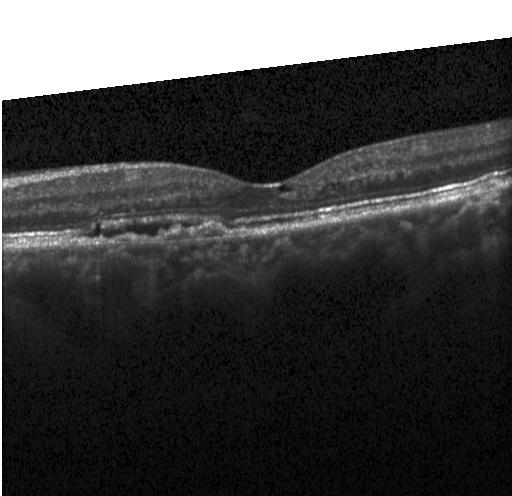 Macular scan; SD-OCT; Heidelberg Spectralis; optical coherence tomography scan. Diagnosis: a choroidal neovascular membrane.